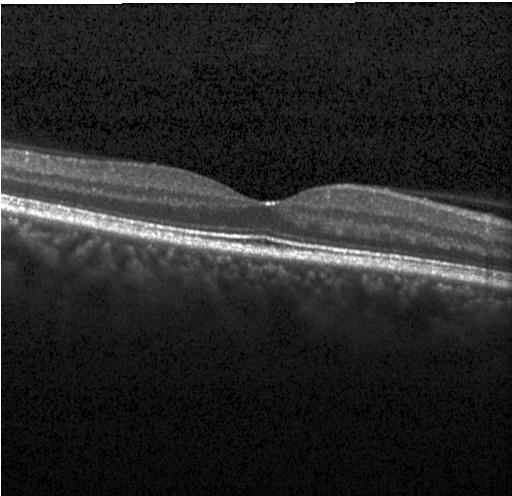 Impression: no choroidal neovascularization, diabetic macular edema, or drusen.